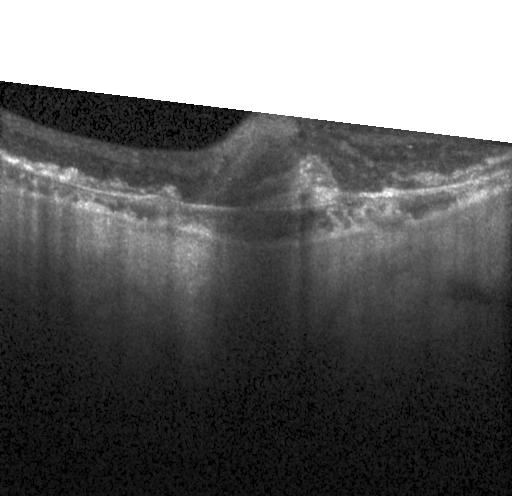 Optical coherence tomography scan; acquired on a Heidelberg Spectralis; SD-OCT; through the macula — This B-scan demonstrates a choroidal neovascular membrane.